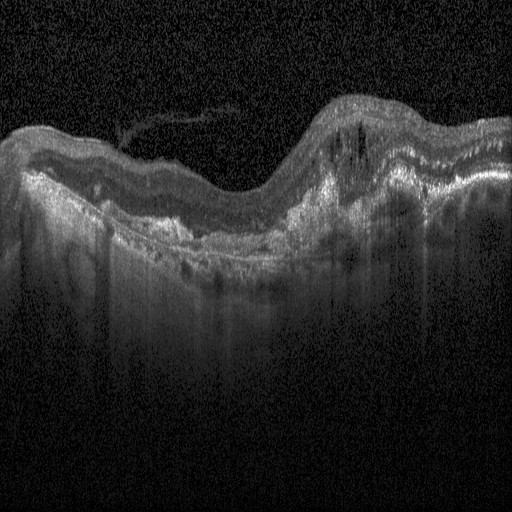 Spectral-domain optical coherence tomography, instrument: Heidelberg Spectralis, OCT line scan. Finding: DME.